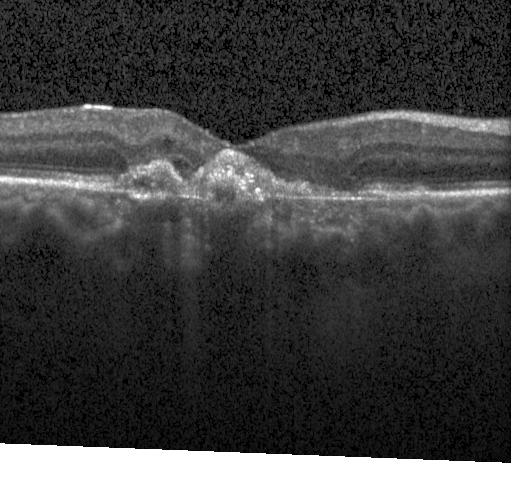 OCT B-scan · centered on the fovea · instrument: Heidelberg Spectralis.
Finding: a choroidal neovascular membrane.